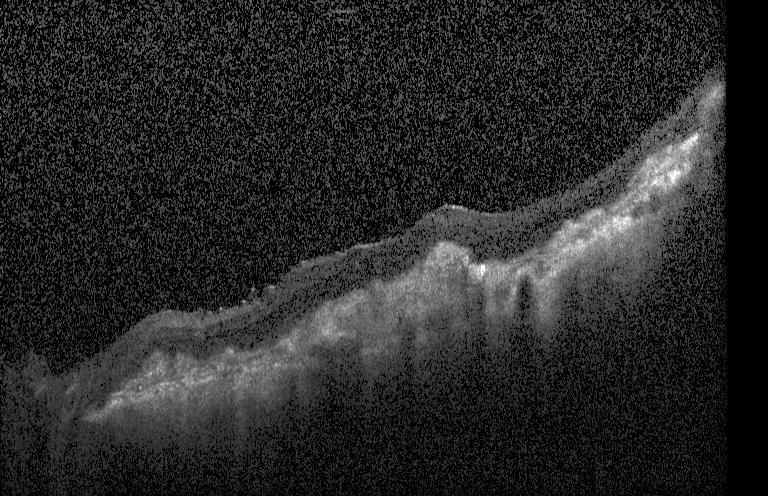
Acquired on a Heidelberg Spectralis. Spectral-domain optical coherence tomography. Macular scan. OCT line scan.
Diagnosis: a choroidal neovascular membrane.